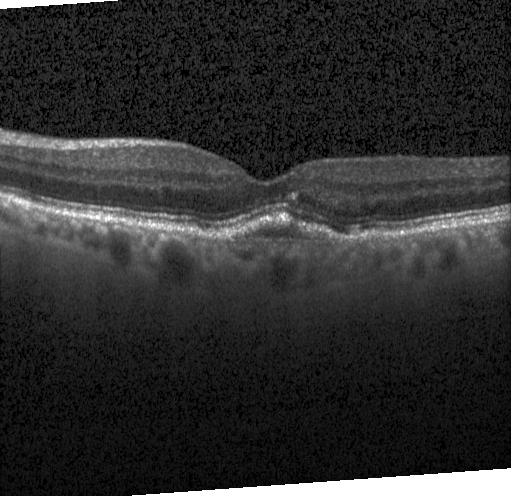 Impression: choroidal neovascularization.